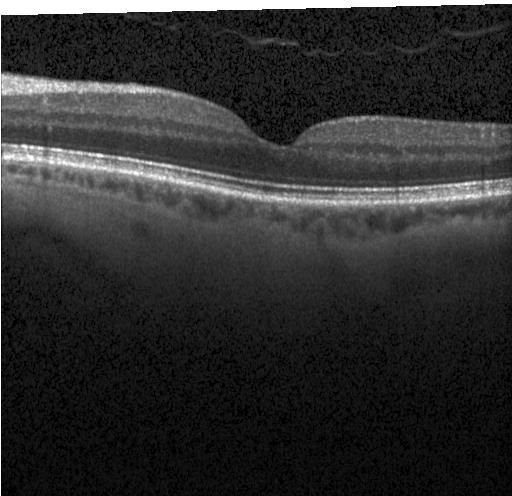 Spectral-domain optical coherence tomography, optical coherence tomography scan — No evidence of CNV, DME, or drusen.